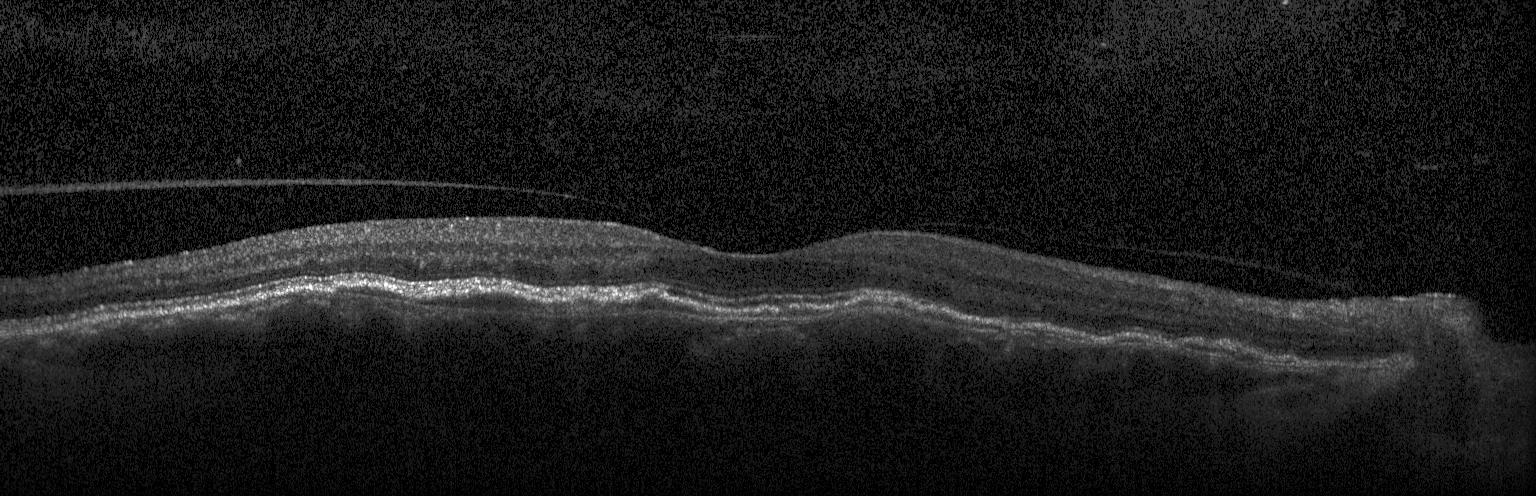 Optical coherence tomography scan; SD-OCT.
Macular OCT: choroidal neovascularization (CNV).